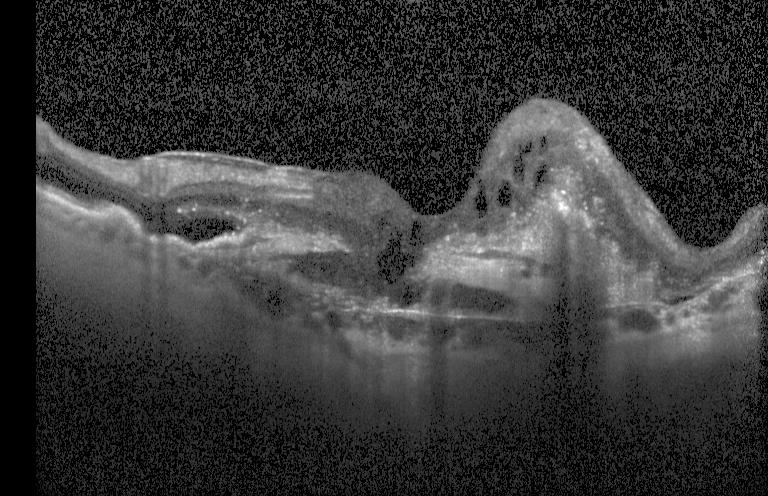
Fovea-centered. Instrument: Heidelberg Spectralis. SD-OCT. Optical coherence tomography B-scan
Impression: CNV.